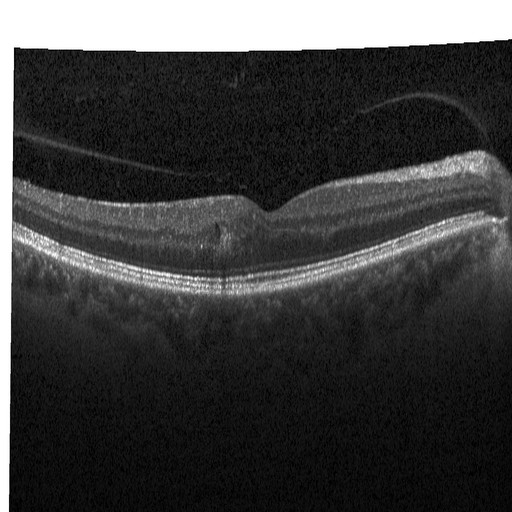
Macular OCT: diabetic macular edema (DME).